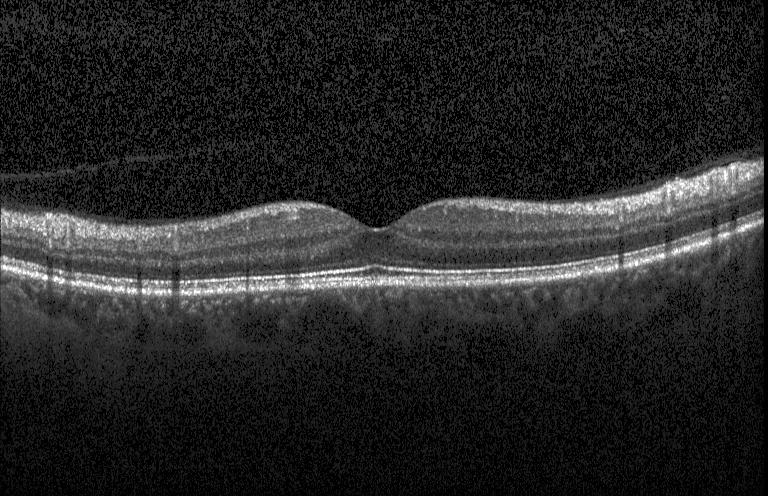
Acquired on a Heidelberg Spectralis. Through the macula. Optical coherence tomography B-scan. Spectral-domain optical coherence tomography.
Impression: no evidence of CNV, DME, or drusen.